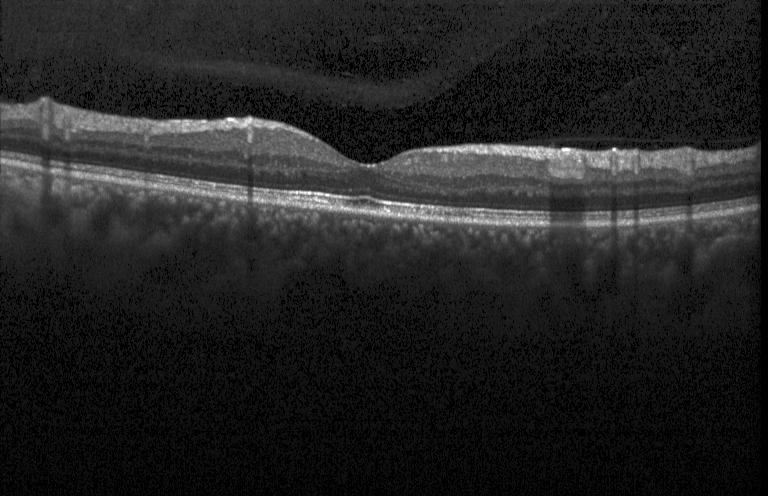 Optical coherence tomography scan. OCT finding: no CNV, no DME, and no drusen.